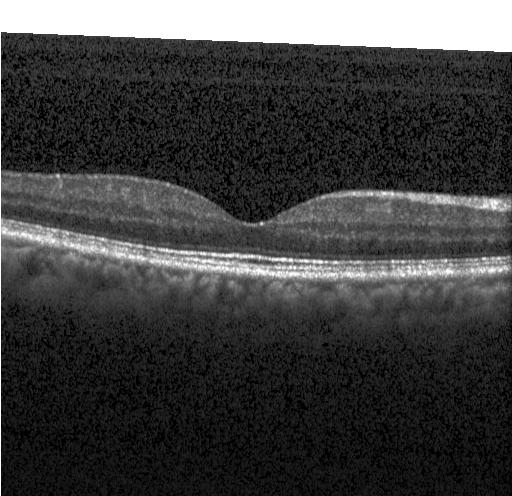

Retinal OCT cross-section showing no choroidal neovascularization, no diabetic macular edema, and no drusen.